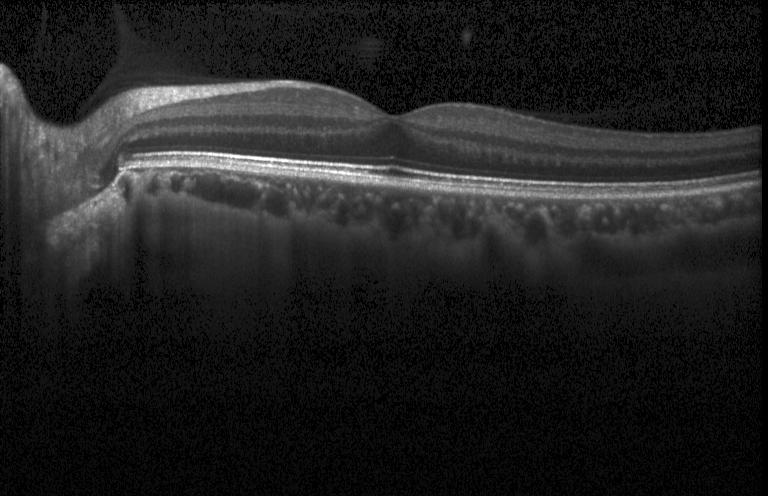 Spectral-domain optical coherence tomography, macular scan, OCT line scan — Dx: no evidence of CNV, DME, or drusen.